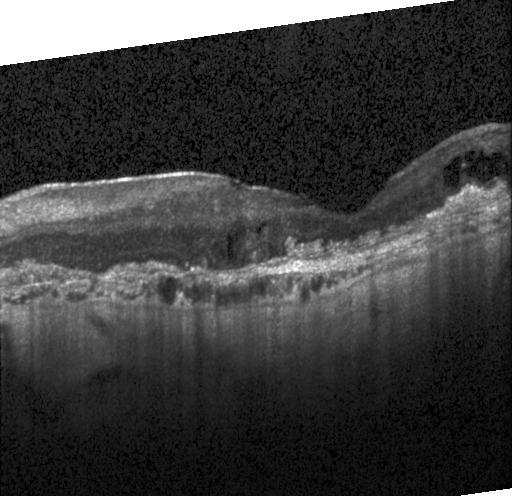

Dx: choroidal neovascularization (CNV).